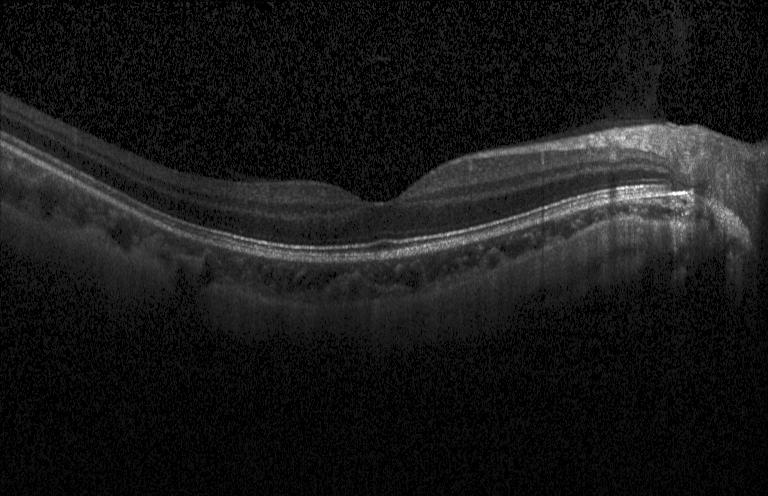 Retinal OCT B-scan. Macular scan. Spectral-domain optical coherence tomography. The scan shows no evidence of CNV, DME, or drusen.